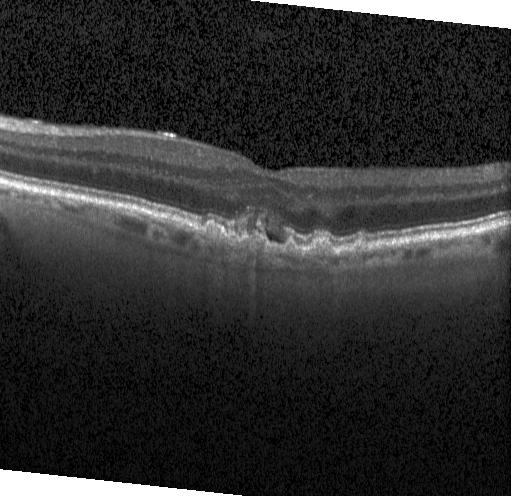 Fovea-centered; retinal OCT cross-section
Impression: choroidal neovascularization (CNV).